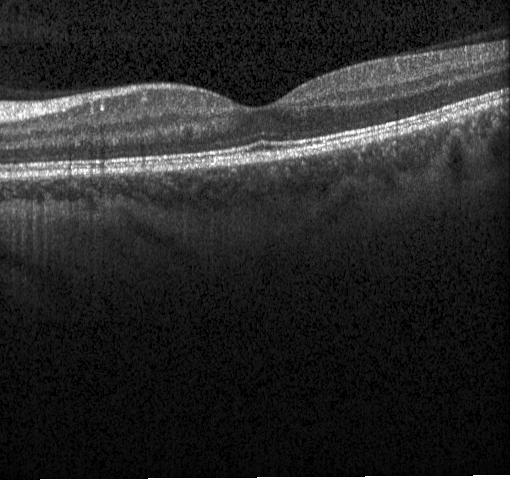 Retinal OCT cross-section showing no choroidal neovascularization, diabetic macular edema, or drusen.